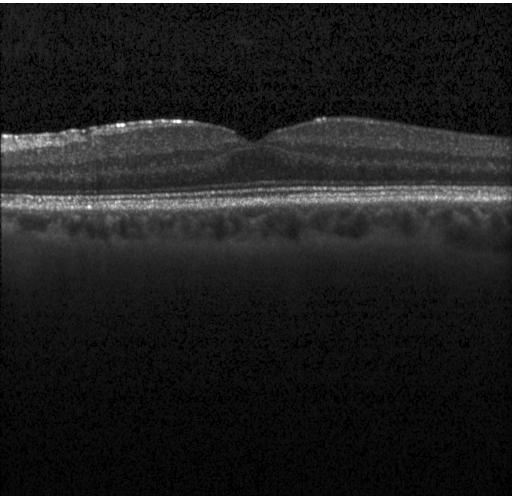 Retinal OCT cross-section · spectral-domain OCT · macular scan · instrument: Heidelberg Spectralis — This B-scan demonstrates no CNV, DME, or drusen.